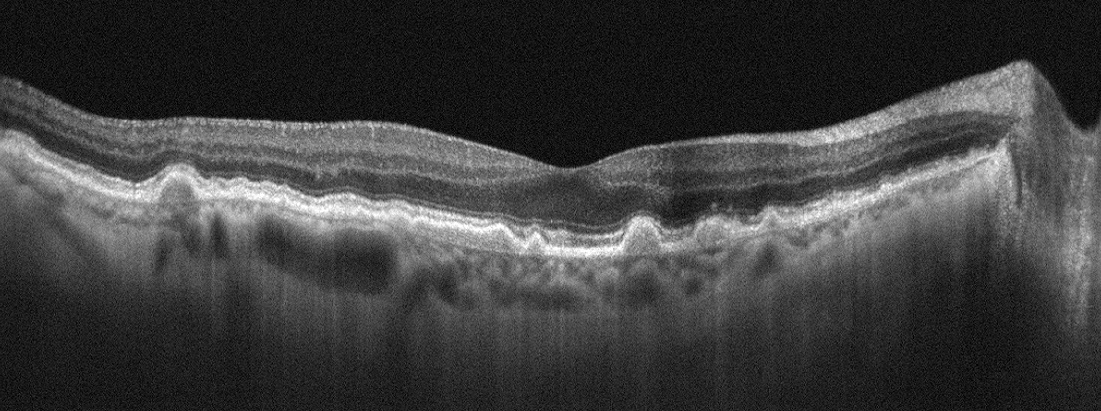 Macular OCT: AMD.